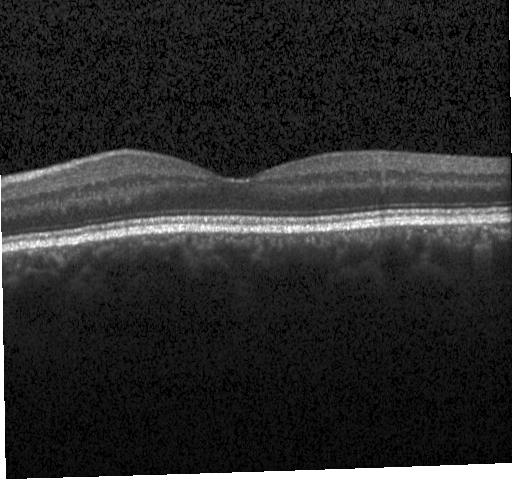
Spectral-domain optical coherence tomography, Heidelberg Spectralis OCT system, fovea-centered, OCT B-scan. The scan shows no choroidal neovascularization, no diabetic macular edema, and no drusen.